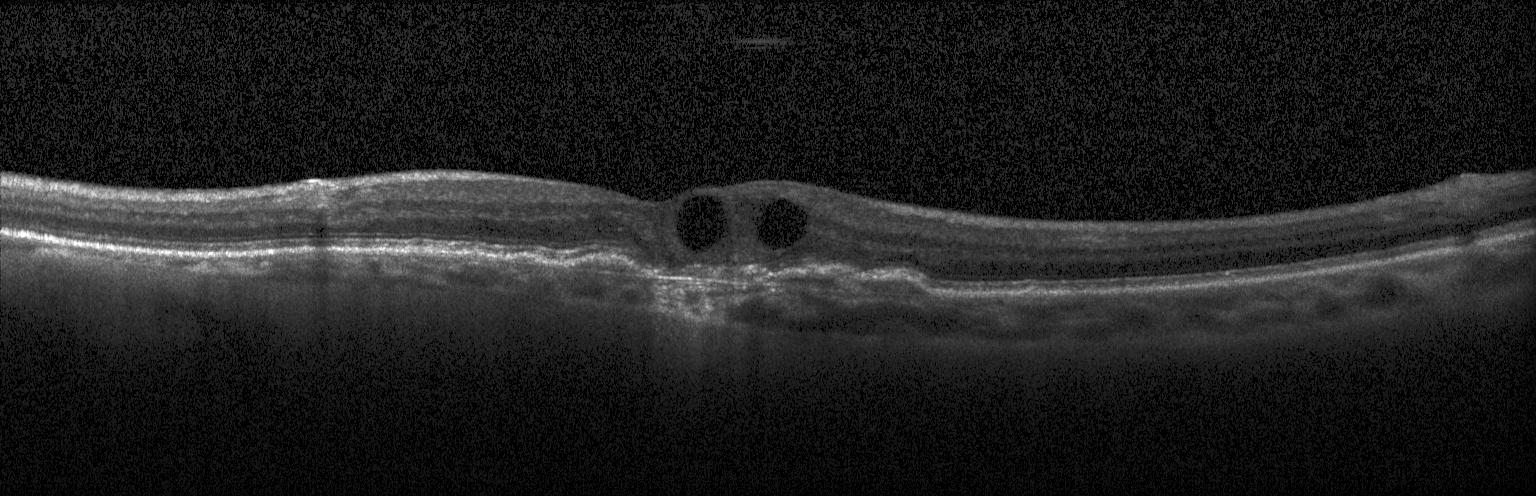
Optical coherence tomography scan. Dx: choroidal neovascularization (CNV).